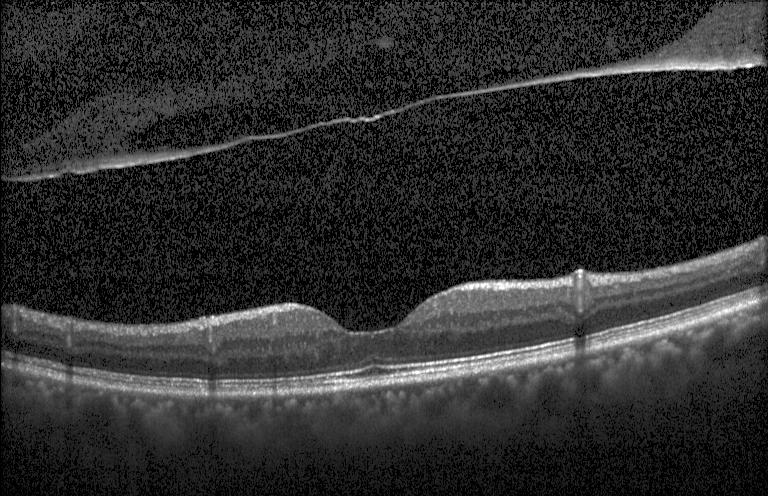
Through the macula · spectral-domain OCT · retinal OCT B-scan
Finding: no evidence of choroidal neovascularization, diabetic macular edema, or drusen.